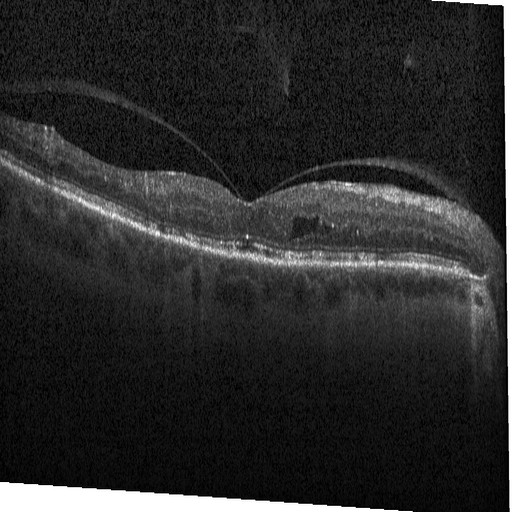

Finding: DME.